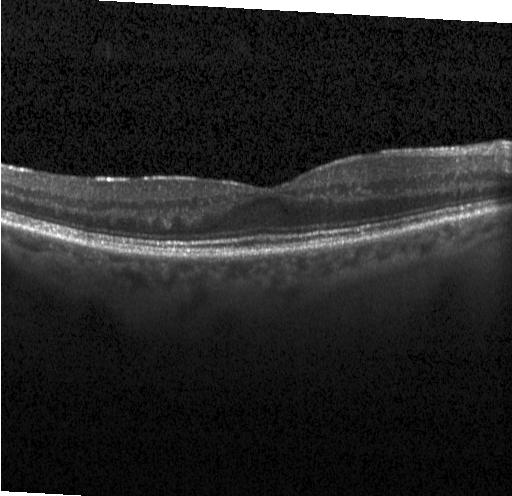
Dx: no choroidal neovascularization, diabetic macular edema, or drusen.